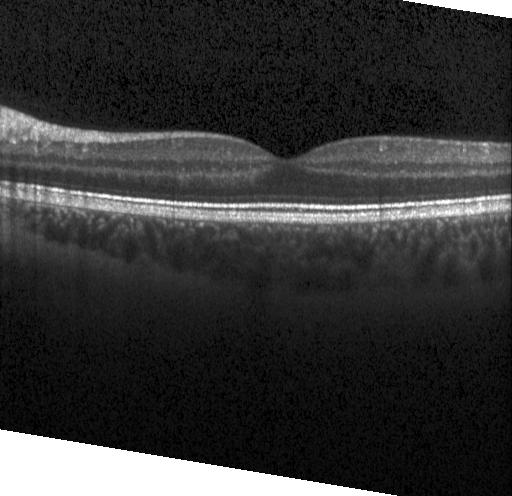

OCT line scan — Diagnosis: no evidence of CNV, DME, or drusen.